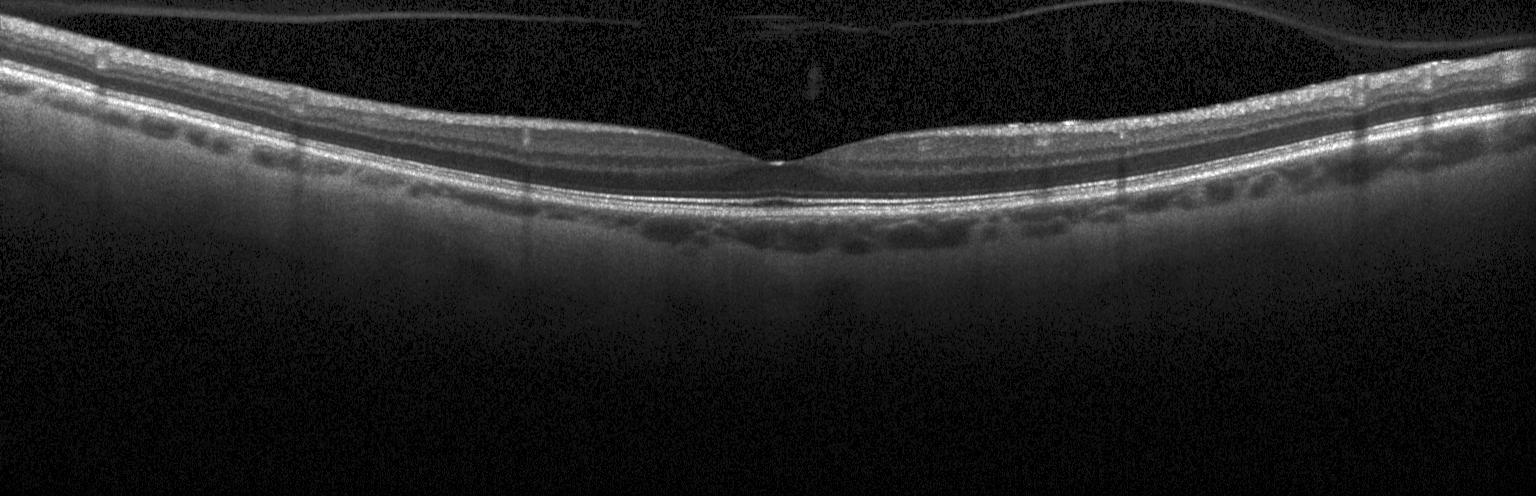

Macular OCT demonstrating neither choroidal neovascularization, diabetic macular edema, nor drusen.